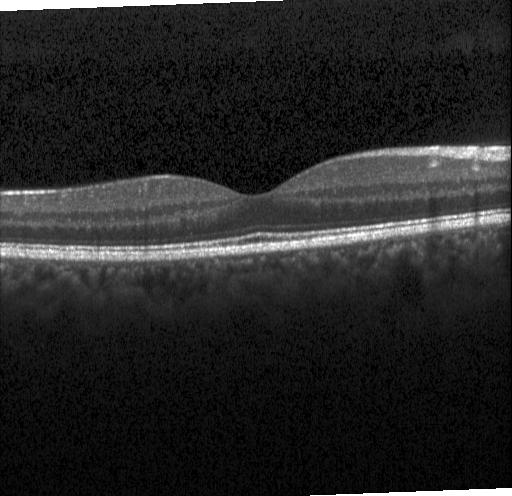

OCT finding: no choroidal neovascularization, diabetic macular edema, or drusen.